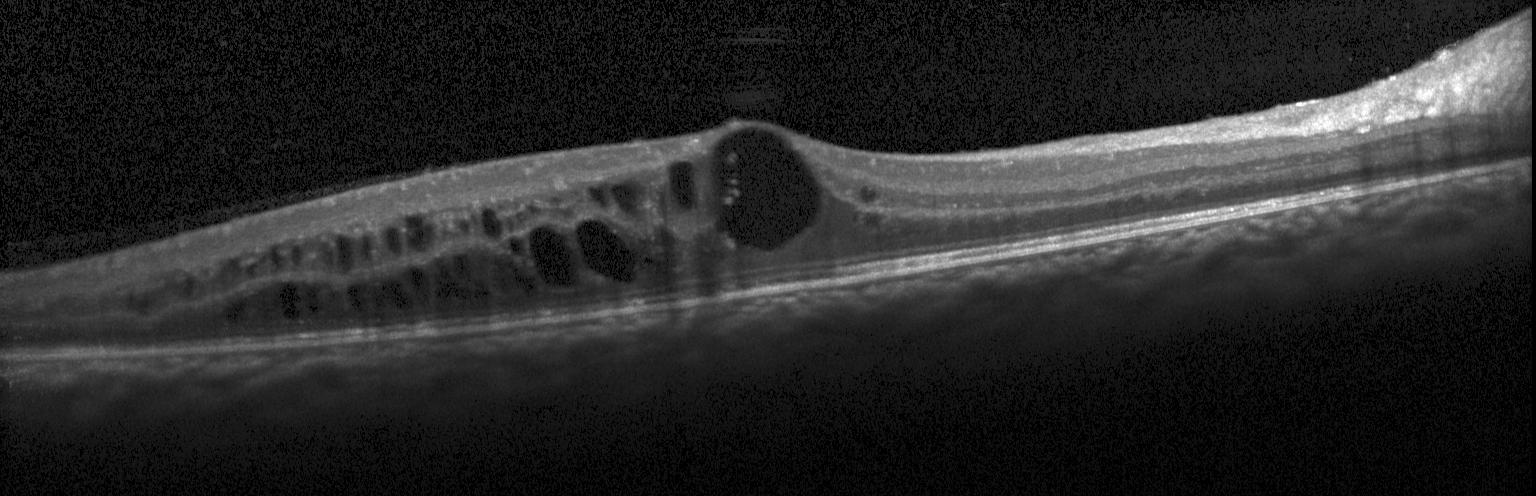

Macular scan. Instrument: Heidelberg Spectralis. OCT line scan.
Diabetic macular edema.